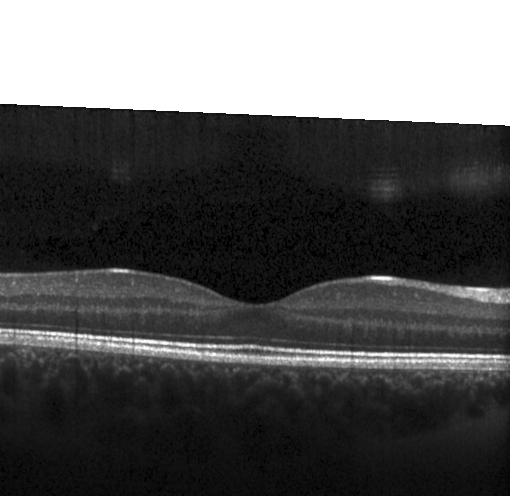 Finding: no evidence of choroidal neovascularization, diabetic macular edema, or drusen.